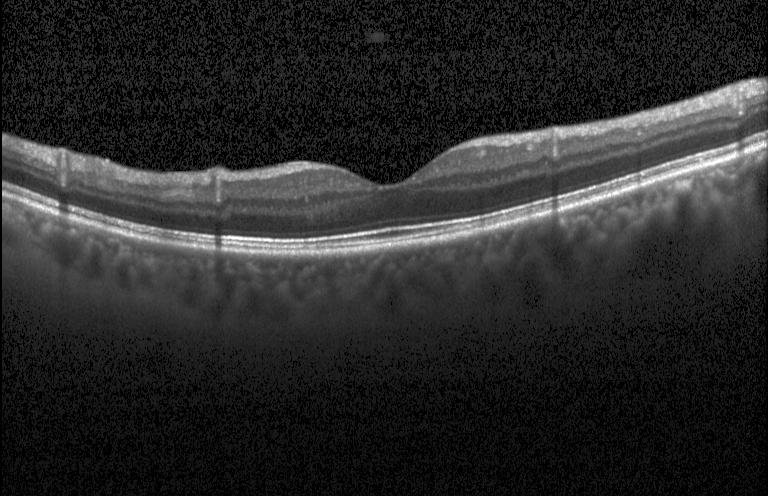
Heidelberg Spectralis OCT system, OCT line scan, fovea-centered. OCT finding: neither CNV, DME, nor drusen.